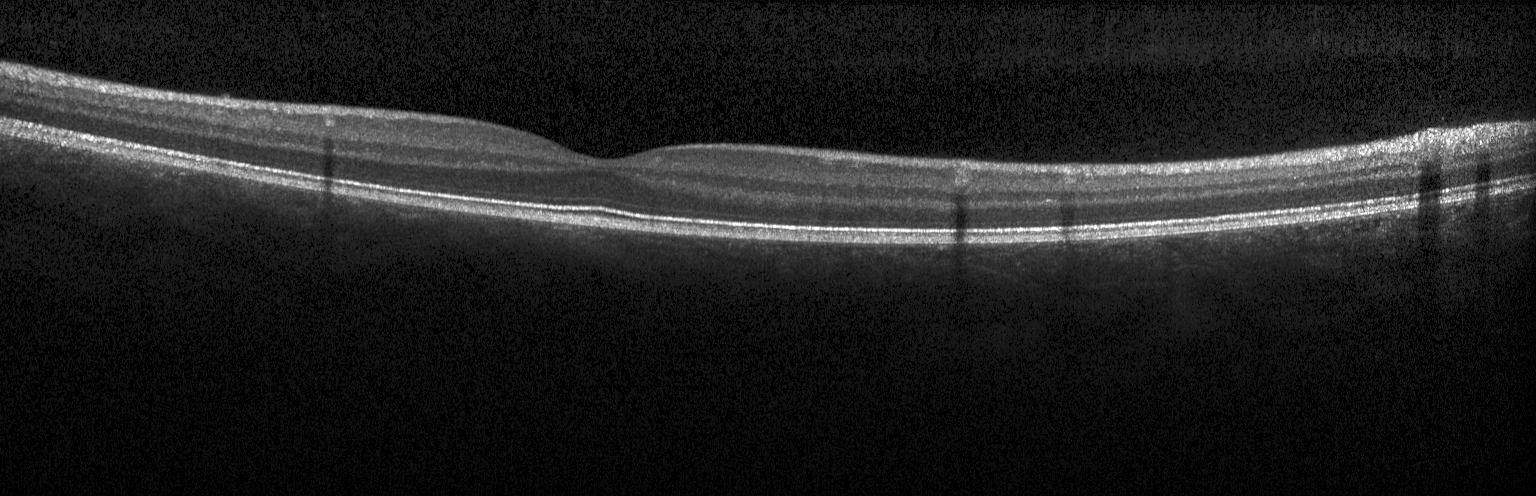 Horizontal scan through the fovea; retinal OCT B-scan; spectral-domain OCT — The scan shows no evidence of choroidal neovascularization, diabetic macular edema, or drusen.